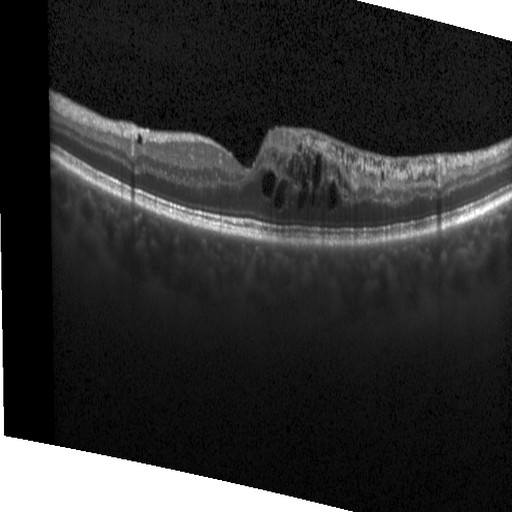
Spectral-domain OCT B-scan: diabetic macular edema.